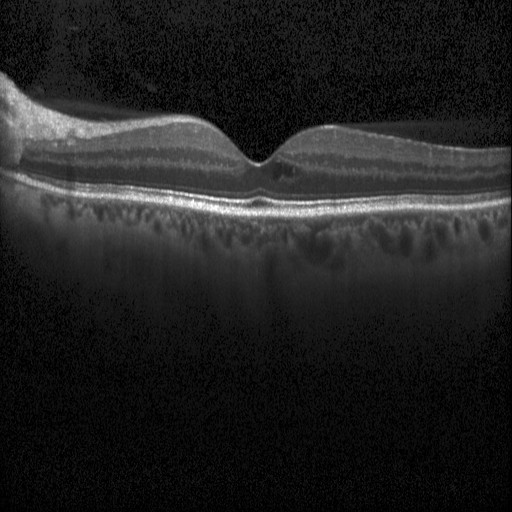

Instrument: Heidelberg Spectralis; retinal OCT cross-section; SD-OCT — OCT finding: diabetic macular edema (DME).